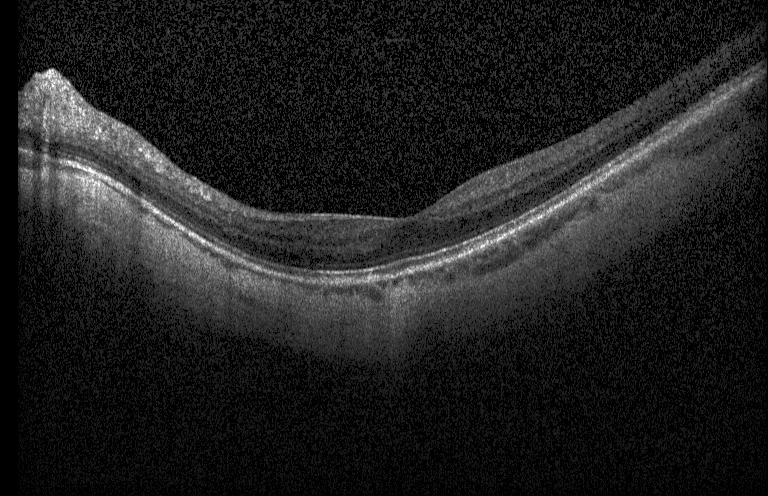 SD-OCT; OCT line scan
Impression: no CNV, no DME, and no drusen.